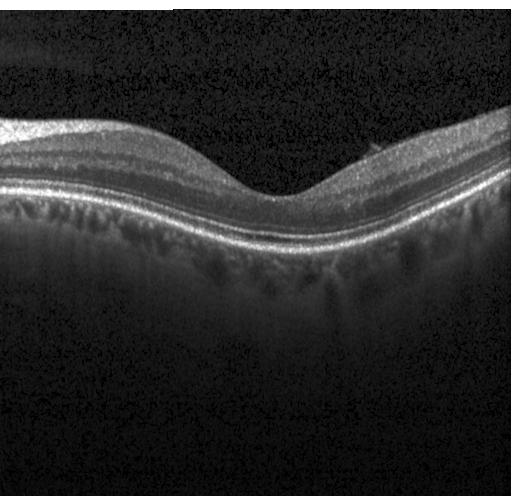
Finding: no choroidal neovascularization, no diabetic macular edema, and no drusen.